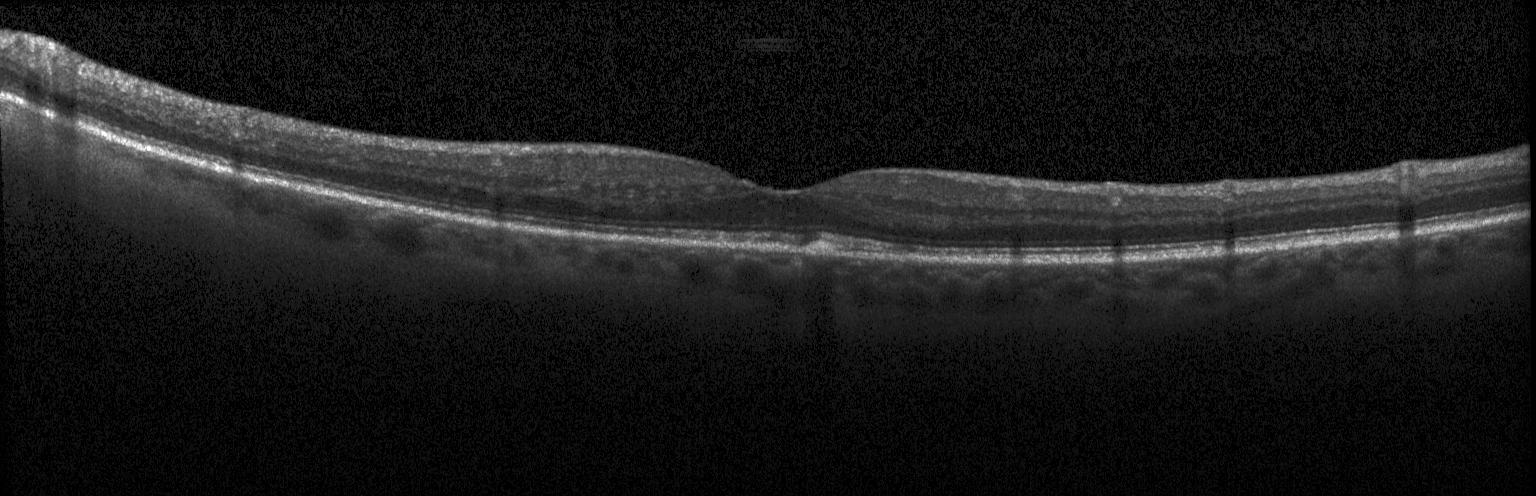

The scan shows multiple drusen.